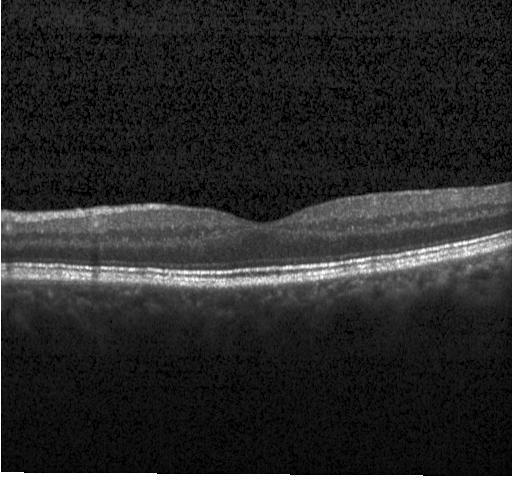 OCT line scan
Diagnosis: no CNV, DME, or drusen.